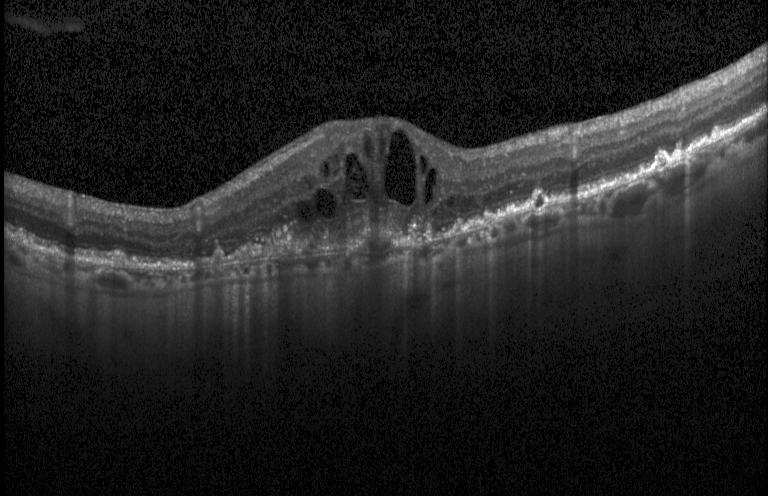

Retinal OCT B-scan. Heidelberg Spectralis OCT system
This B-scan demonstrates a choroidal neovascular membrane.